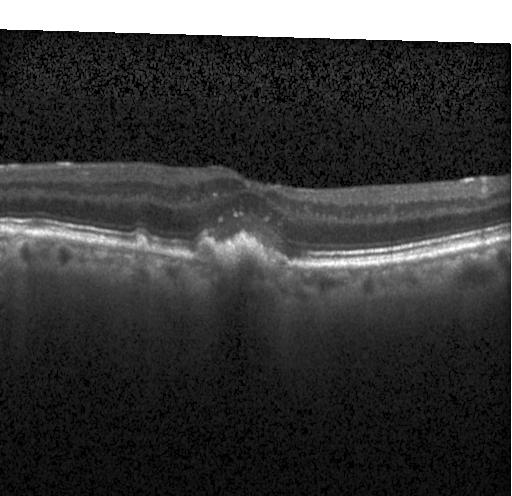
Retinal OCT cross-section; acquired on a Heidelberg Spectralis
Macular OCT: a choroidal neovascular membrane.